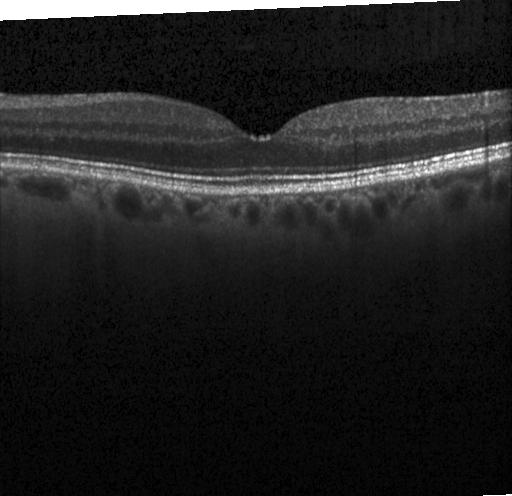
Impression: no choroidal neovascularization, no diabetic macular edema, and no drusen.